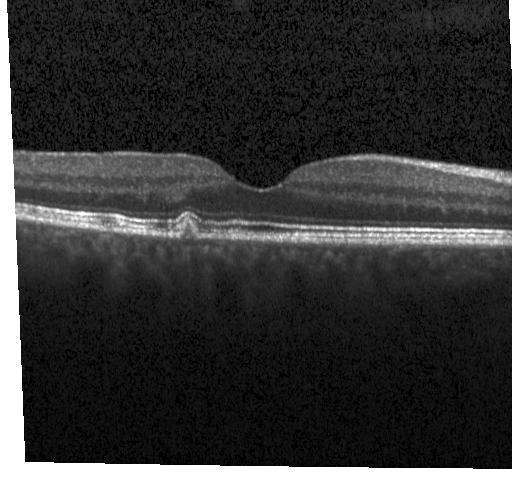

The scan shows sub-RPE drusenoid deposits.